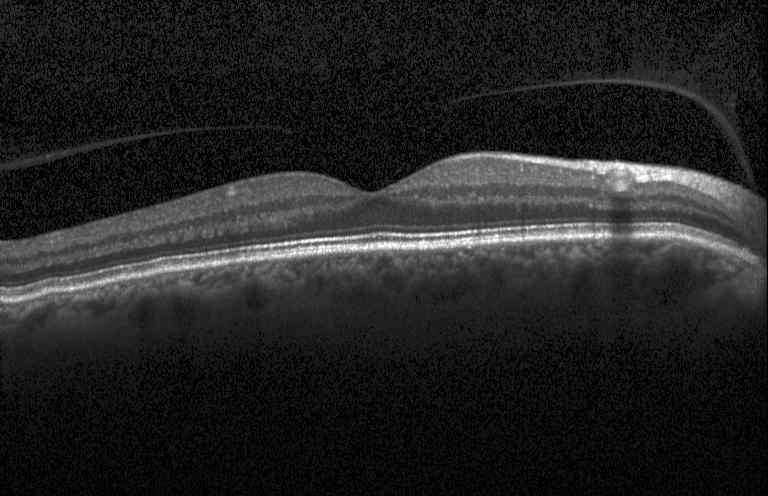
Spectral-domain OCT · OCT B-scan · through the macula · Heidelberg Spectralis
The scan shows no choroidal neovascularization, no diabetic macular edema, and no drusen.